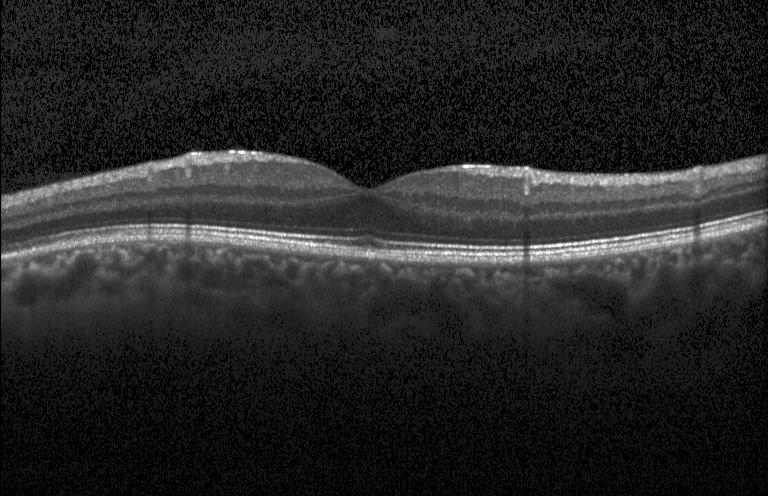
OCT B-scan.
Diagnosis: neither choroidal neovascularization, diabetic macular edema, nor drusen.